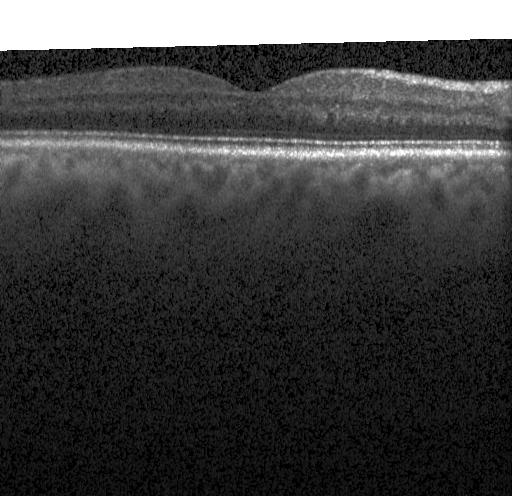
Dx: no choroidal neovascularization, no diabetic macular edema, and no drusen.